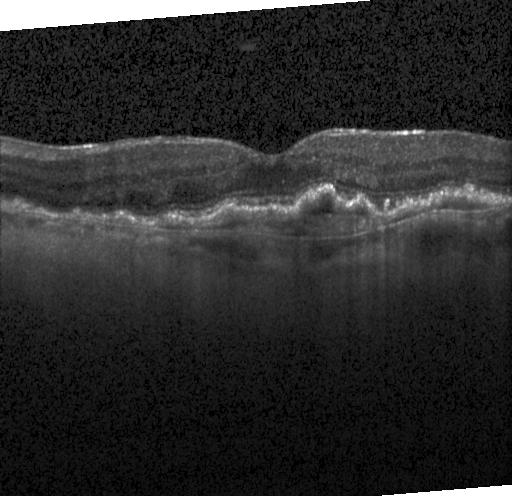
Heidelberg Spectralis OCT system, optical coherence tomography B-scan.
Diagnosis: choroidal neovascularization.